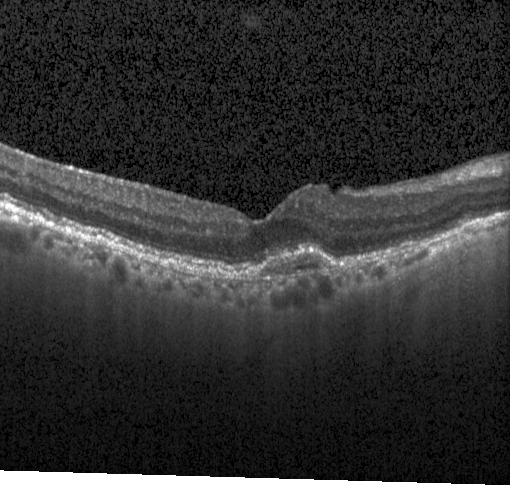 Optical coherence tomography scan · fovea-centered · spectral-domain optical coherence tomography. Dx: CNV.